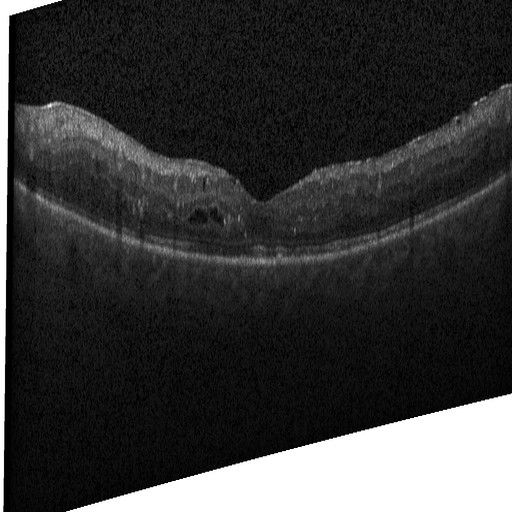

Retinal OCT B-scan; spectral-domain OCT. Diabetic macular edema.